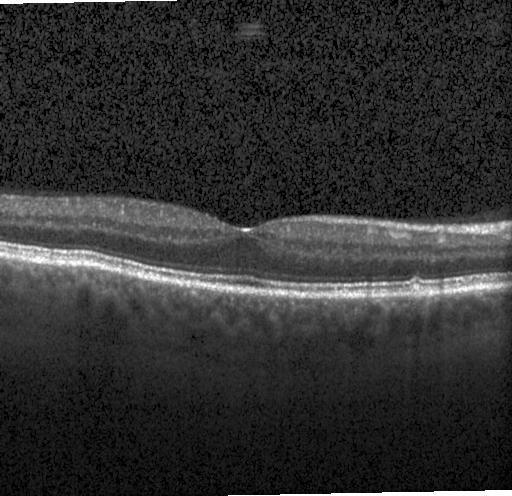
Finding: no evidence of choroidal neovascularization, diabetic macular edema, or drusen.